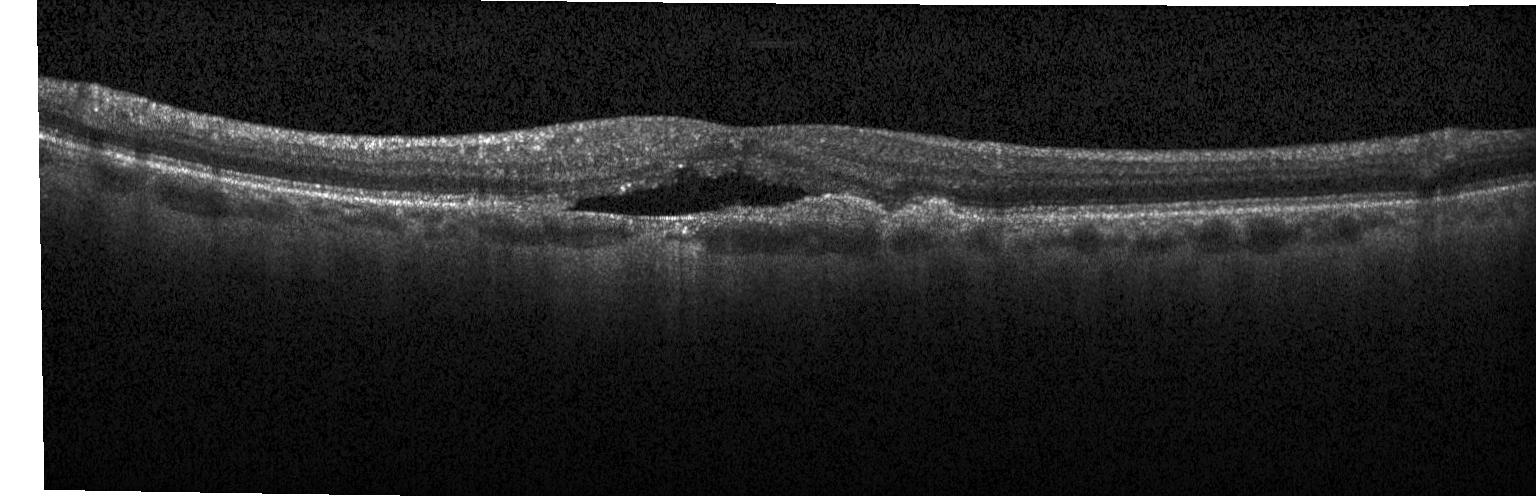 OCT finding: choroidal neovascularization.